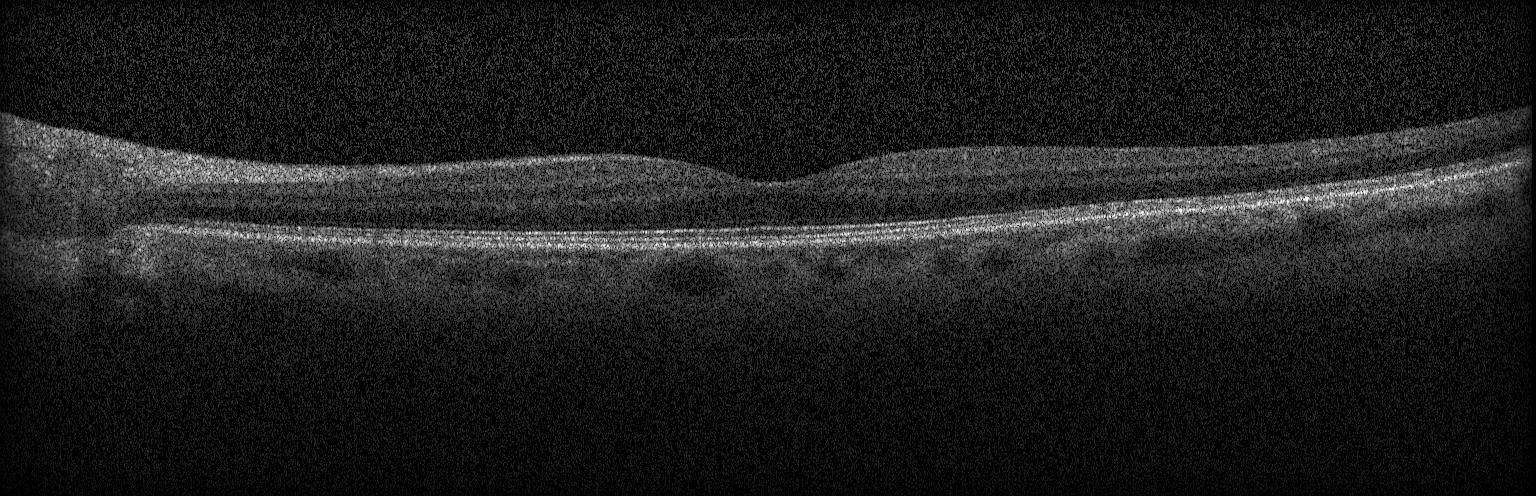

The scan shows neither choroidal neovascularization, diabetic macular edema, nor drusen.